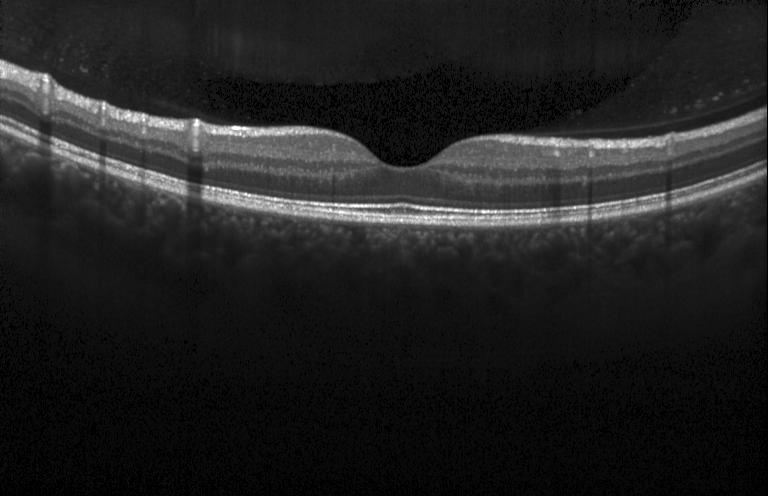
Spectral-domain OCT, acquired on a Heidelberg Spectralis, OCT line scan, through the macula.
No choroidal neovascularization, diabetic macular edema, or drusen.